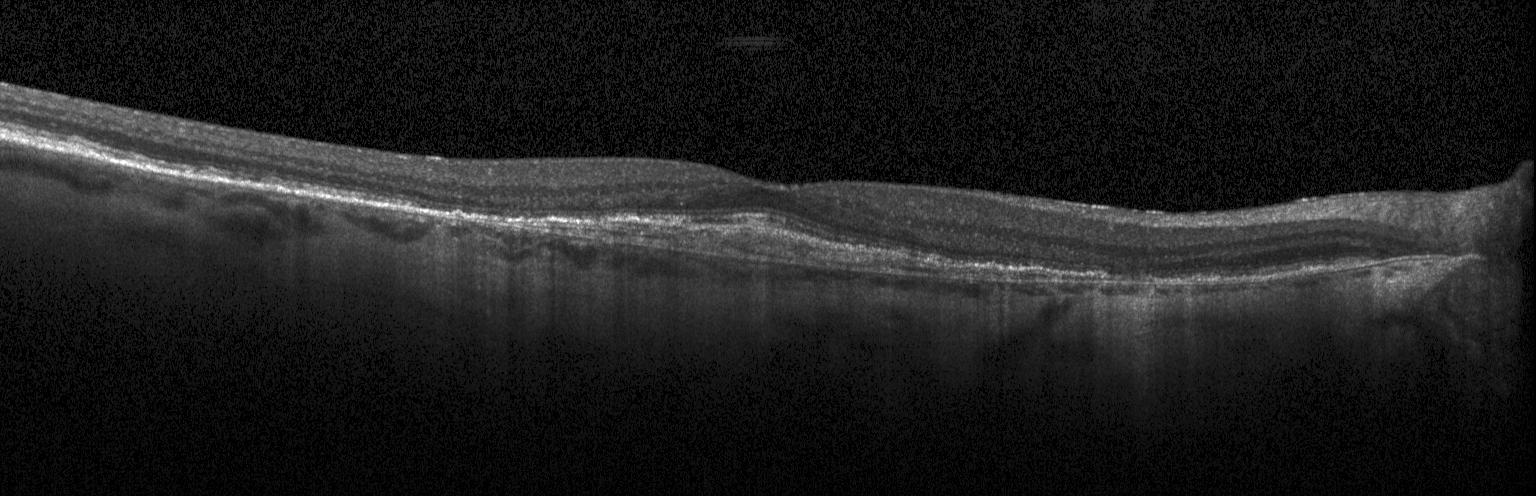
OCT B-scan. Assessment: a choroidal neovascular membrane.